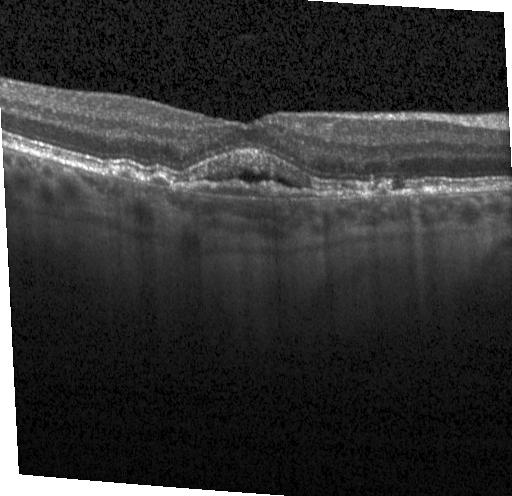
Finding: a choroidal neovascular membrane.